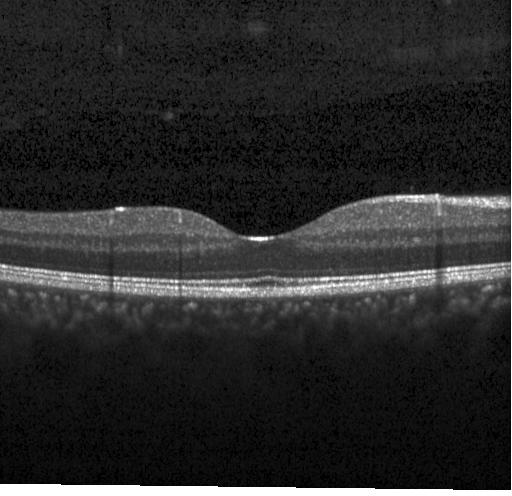
Impression: neither CNV, DME, nor drusen.